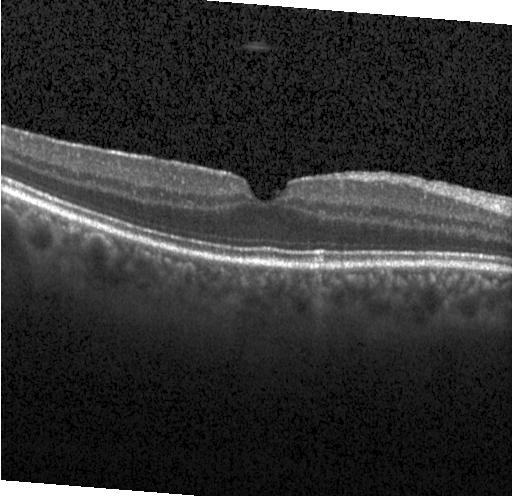
Diagnosis: no choroidal neovascularization, no diabetic macular edema, and no drusen.